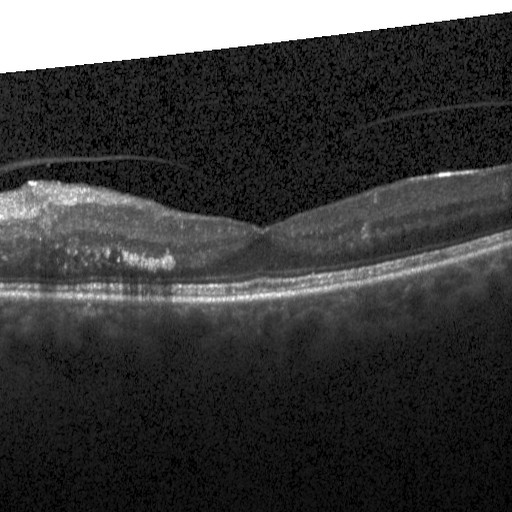

Dx: DME.